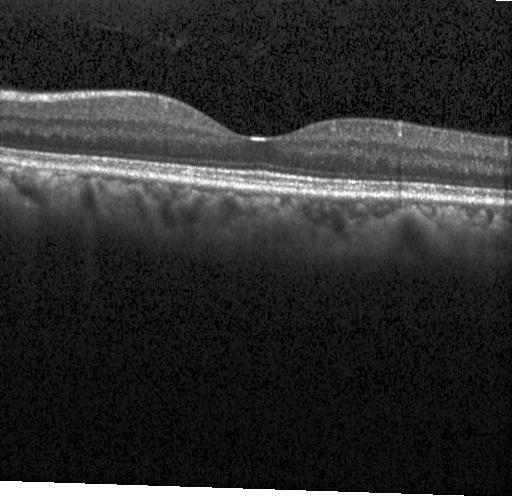

Optical coherence tomography B-scan. Macular scan. Acquired on a Heidelberg Spectralis — Impression: no evidence of choroidal neovascularization, diabetic macular edema, or drusen.